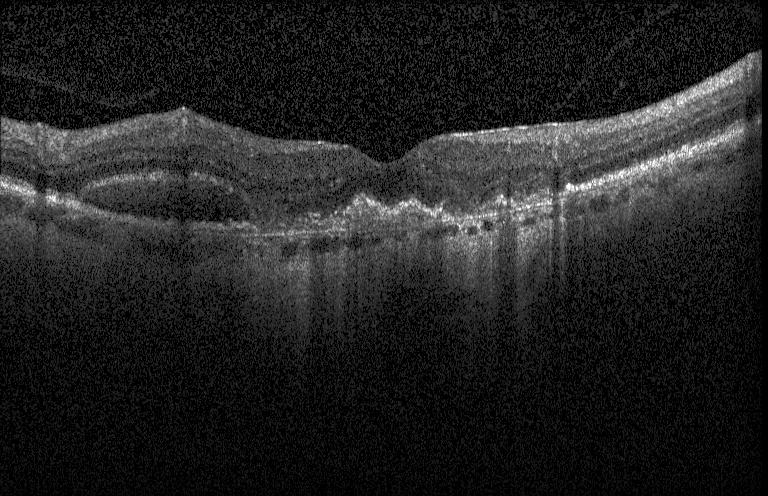

Diagnosis: choroidal neovascularization.